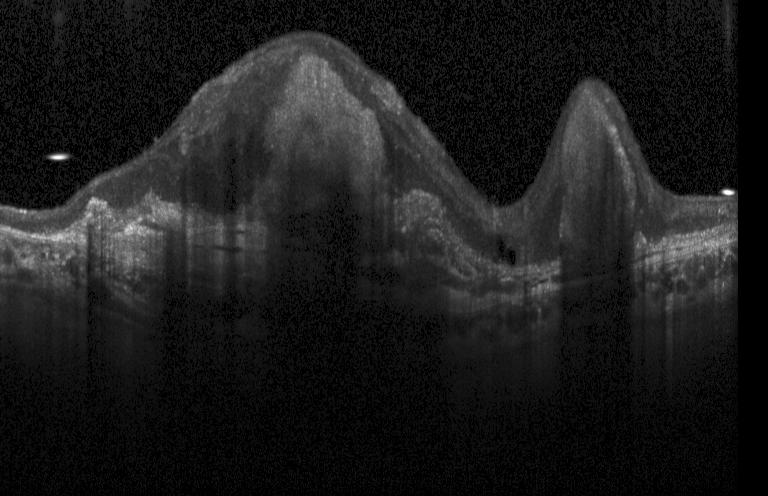

Retinal OCT B-scan · SD-OCT. OCT finding: CNV.